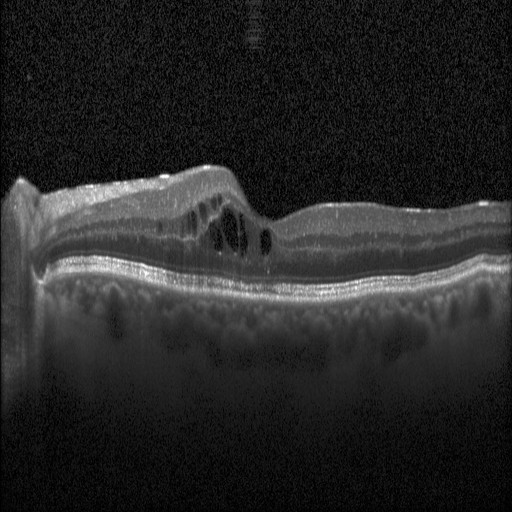
Finding: DME.